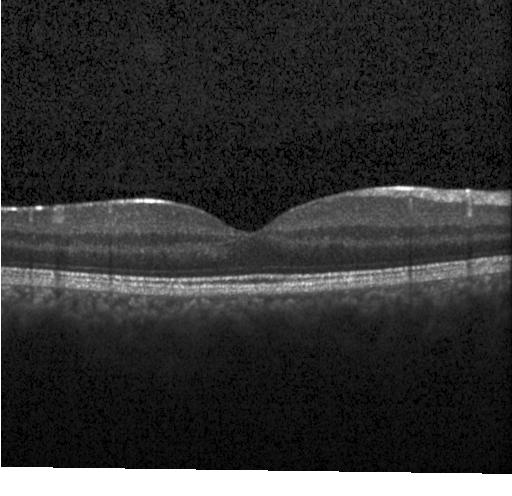

Spectral-domain optical coherence tomography, retinal OCT cross-section, instrument: Heidelberg Spectralis
Neither choroidal neovascularization, diabetic macular edema, nor drusen.